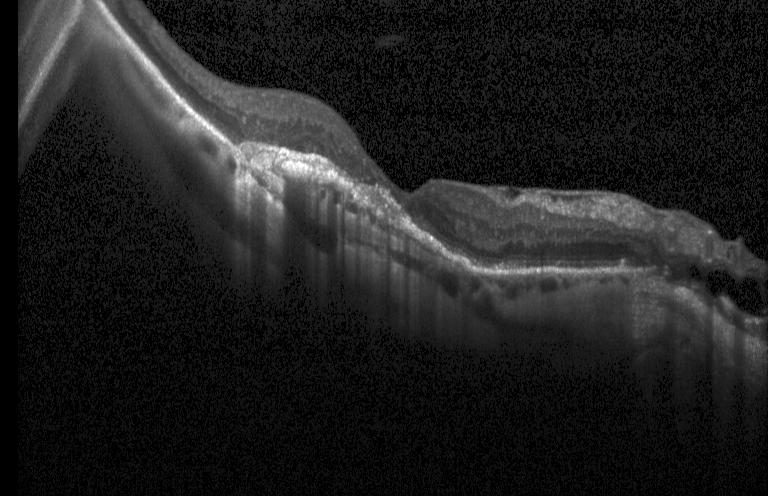 Diagnosis: choroidal neovascularization (CNV).